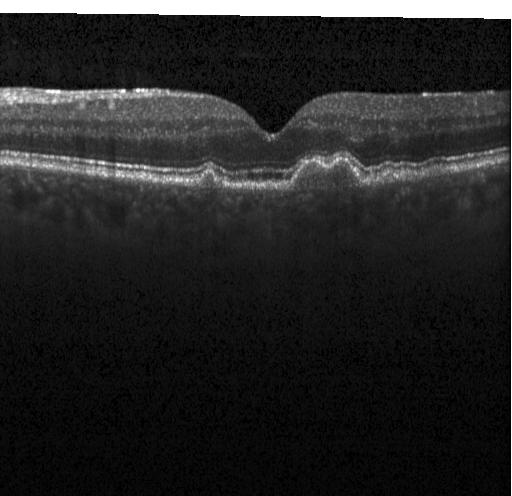
Finding: drusen.